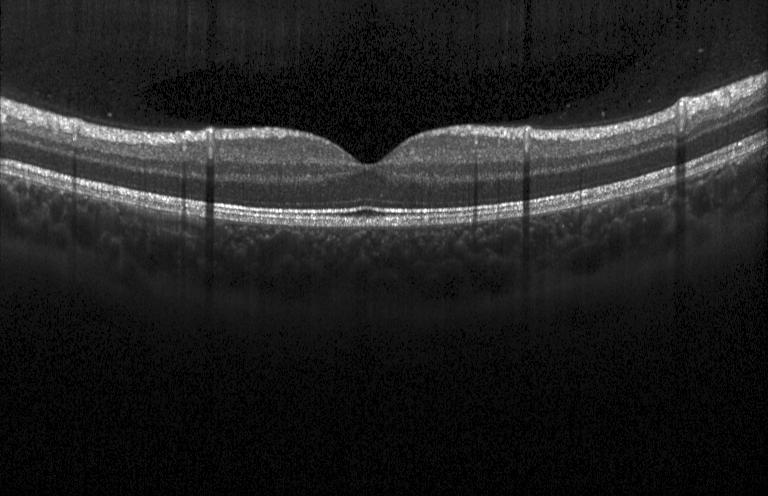
Optical coherence tomography scan · through the macula · Heidelberg Spectralis · SD-OCT — Diagnosis: no evidence of choroidal neovascularization, diabetic macular edema, or drusen.